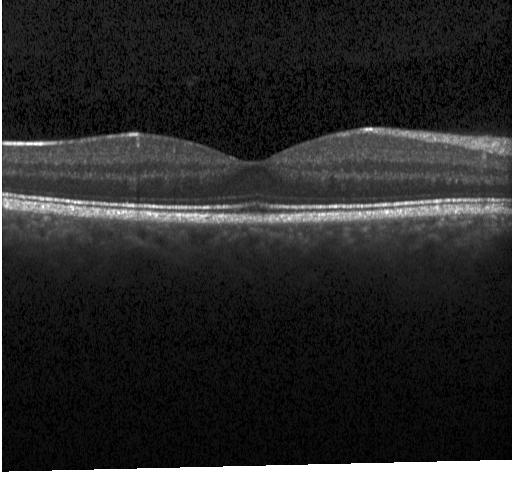

OCT B-scan showing no evidence of choroidal neovascularization, diabetic macular edema, or drusen.